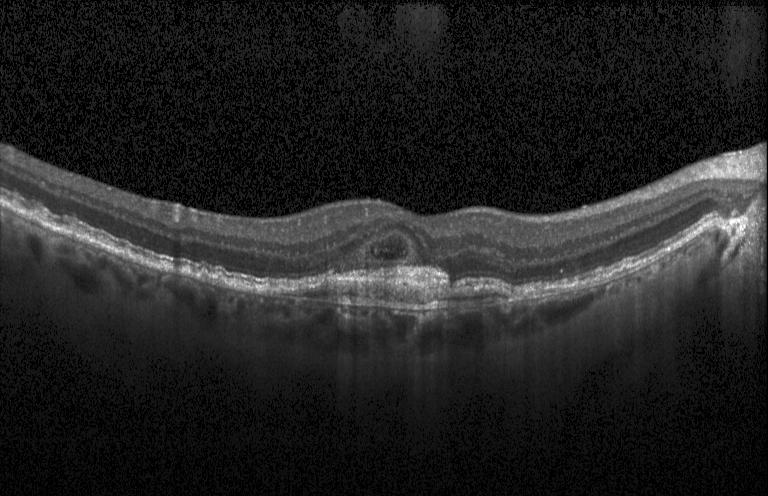
Assessment: a choroidal neovascular membrane.